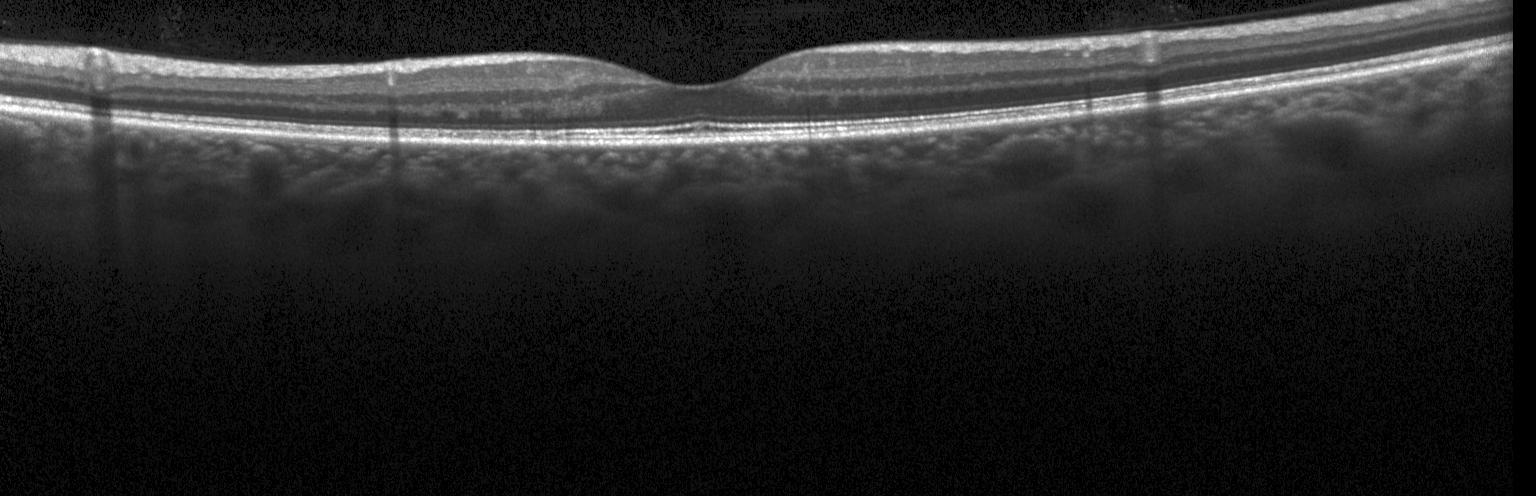
Retinal OCT cross-section showing neither choroidal neovascularization, diabetic macular edema, nor drusen.